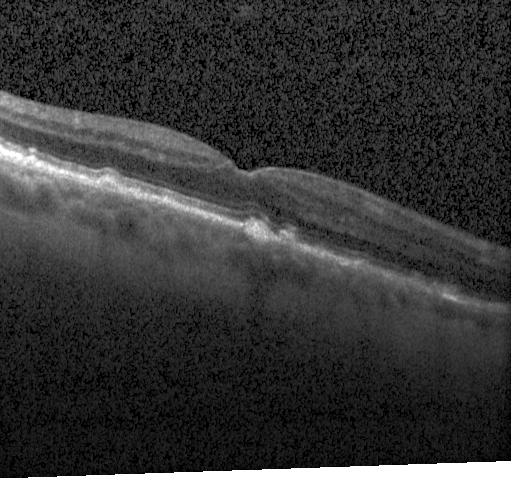

Optical coherence tomography B-scan; spectral-domain optical coherence tomography — Diagnosis: multiple drusen.